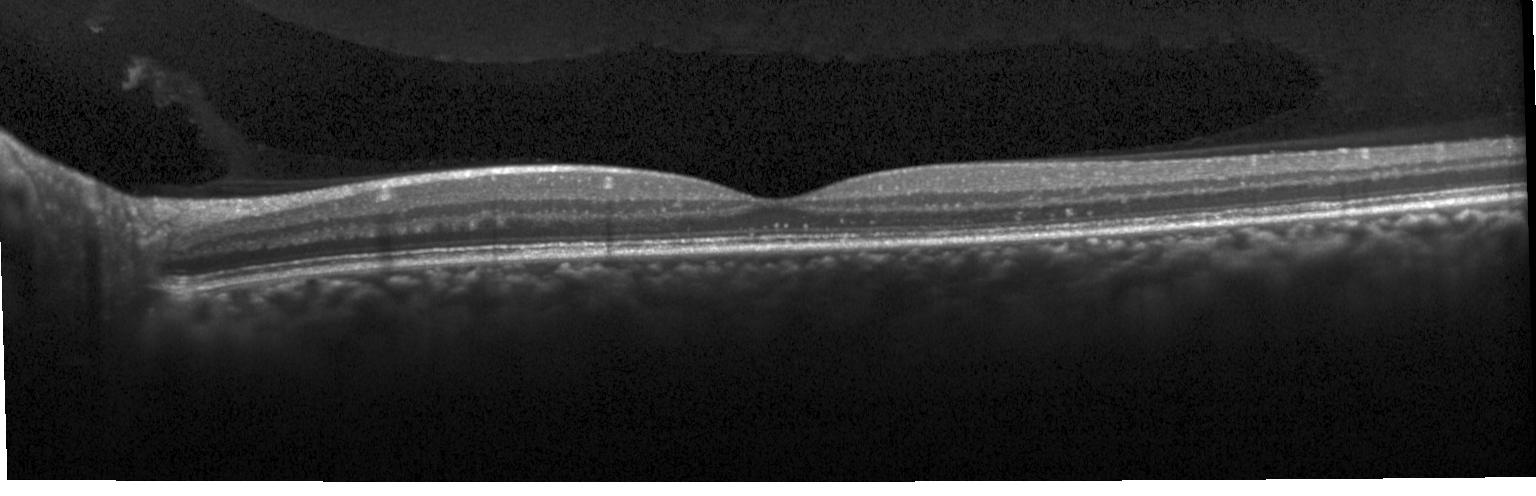

Dx: neither choroidal neovascularization, diabetic macular edema, nor drusen.